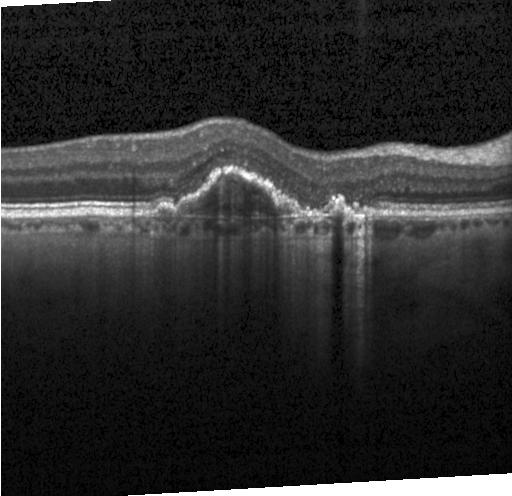

Retinal OCT cross-section showing choroidal neovascularization.